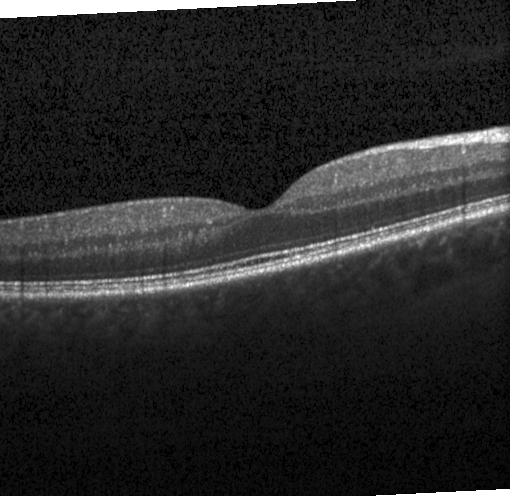

Retinal OCT cross-section showing no evidence of CNV, DME, or drusen.